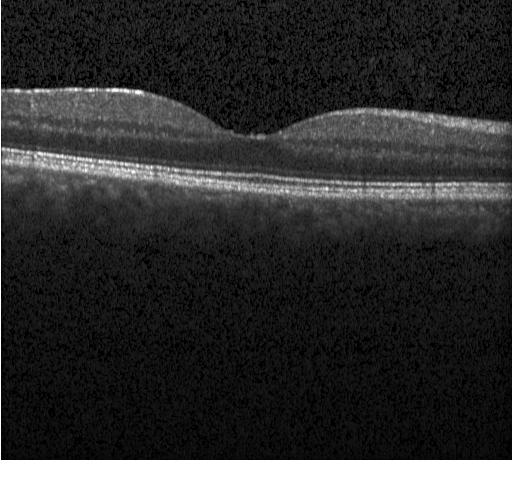

OCT B-scan.
This B-scan demonstrates no CNV, no DME, and no drusen.